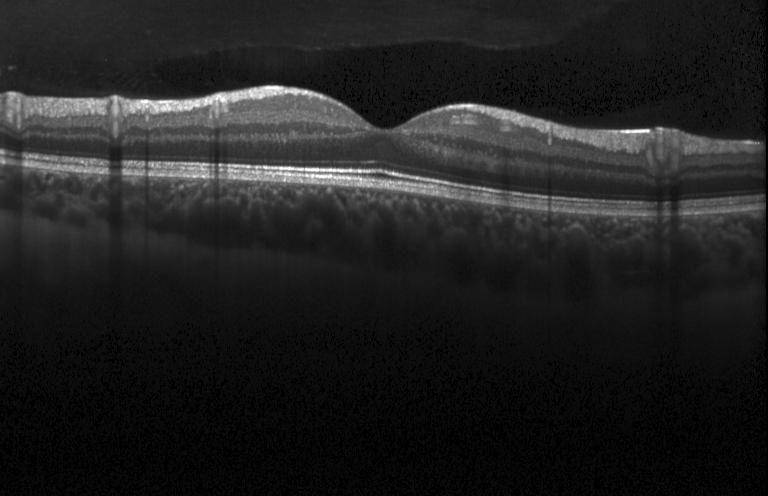
OCT line scan
No choroidal neovascularization, diabetic macular edema, or drusen.